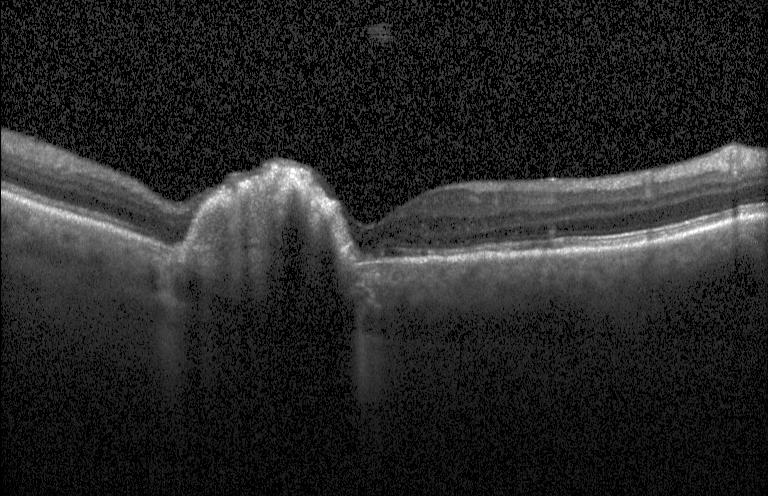 OCT line scan. Dx: choroidal neovascularization.